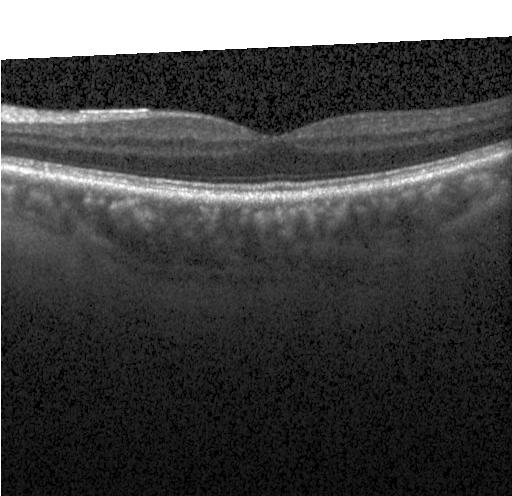
OCT B-scan. The scan shows no evidence of choroidal neovascularization, diabetic macular edema, or drusen.